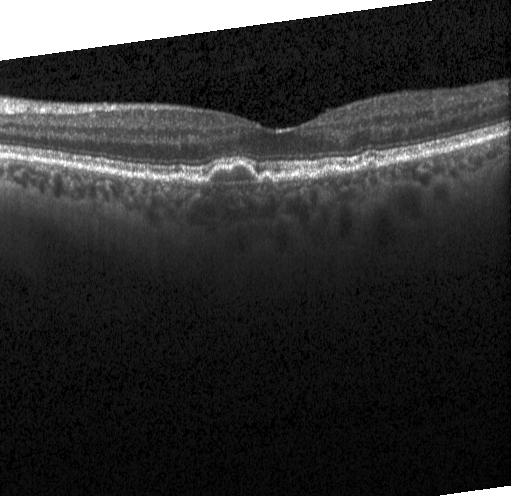
OCT finding: sub-RPE drusenoid deposits.